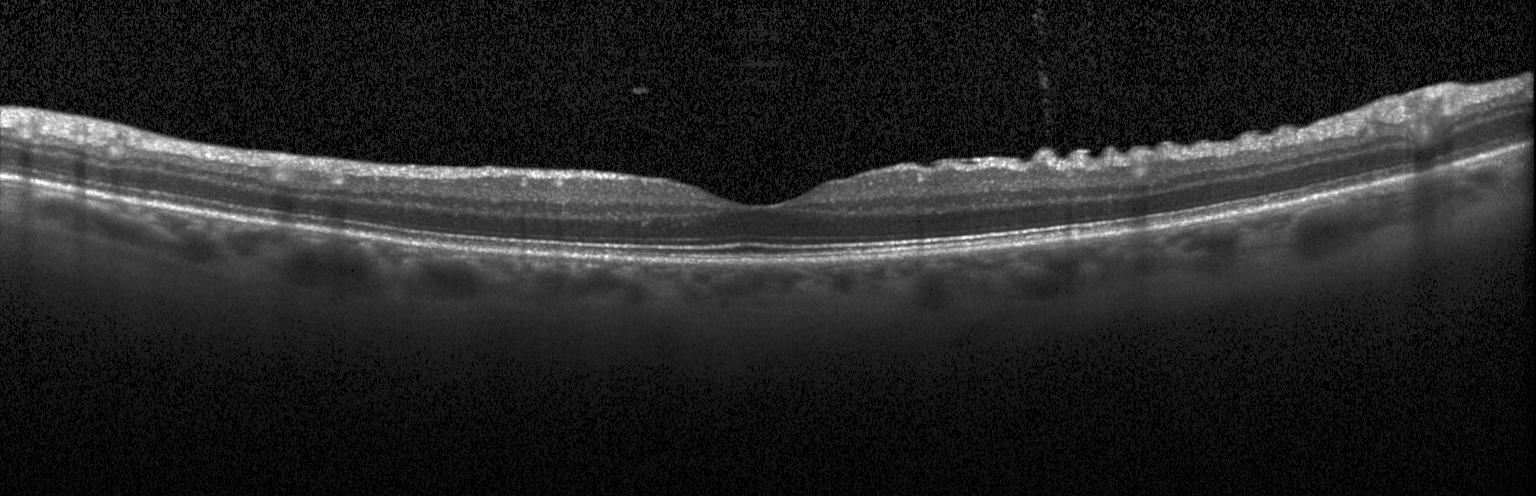
Acquired on a Heidelberg Spectralis. OCT B-scan. Horizontal scan through the fovea
Macular OCT: neither choroidal neovascularization, diabetic macular edema, nor drusen.